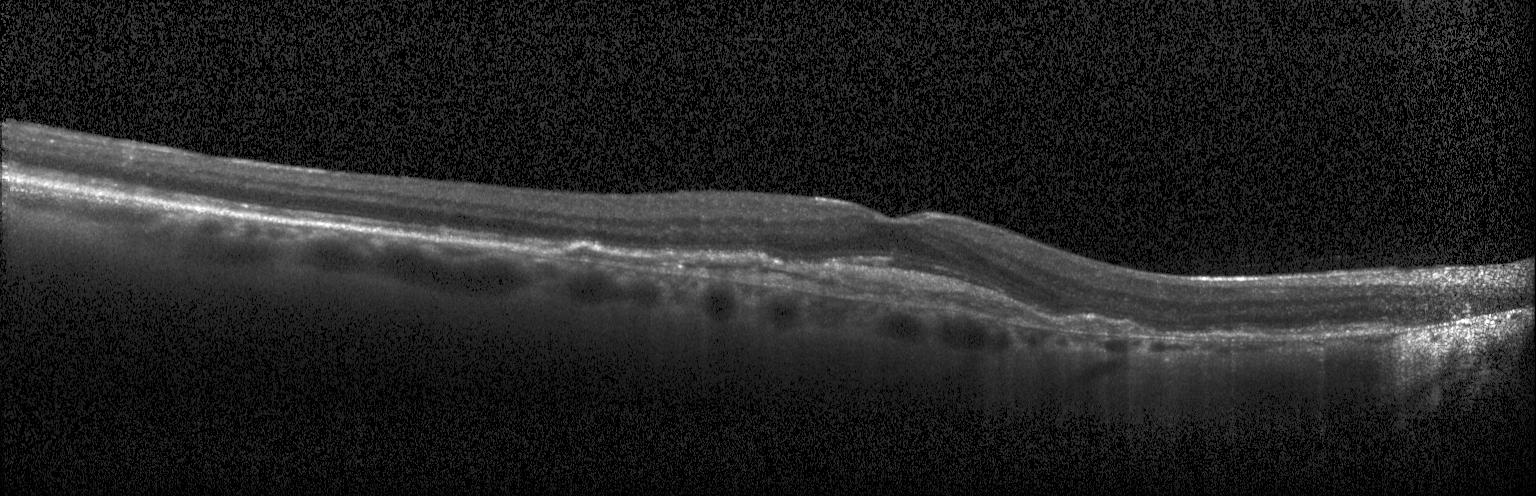 OCT scan showing choroidal neovascularization (CNV).